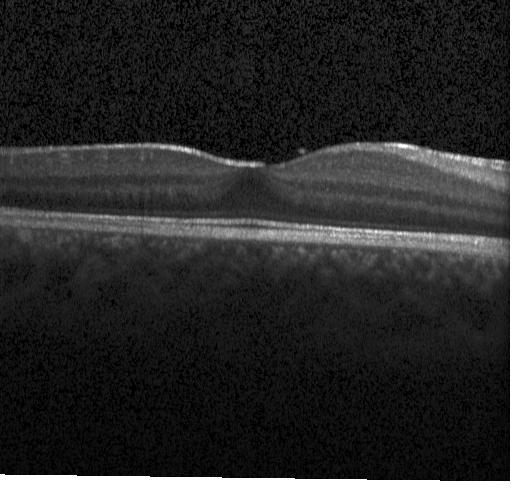
Macular scan. Instrument: Heidelberg Spectralis. SD-OCT. OCT line scan. Dx: no evidence of choroidal neovascularization, diabetic macular edema, or drusen.